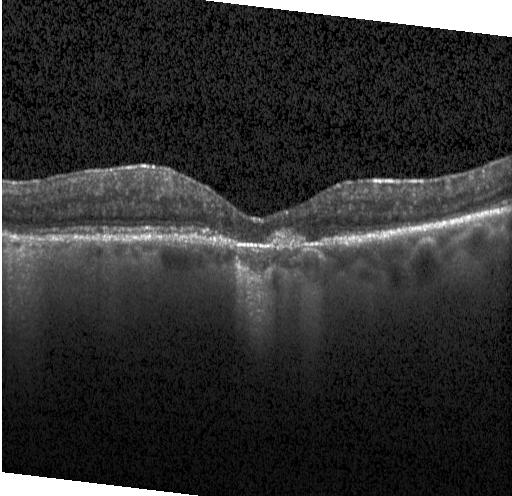
Retinal OCT B-scan
This B-scan demonstrates a choroidal neovascular membrane.